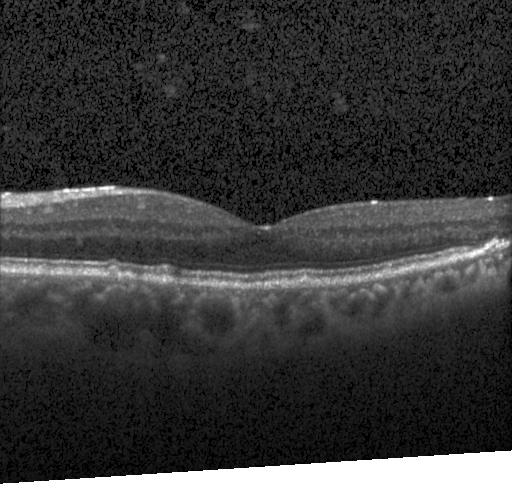

OCT line scan. Diagnosis: drusen.